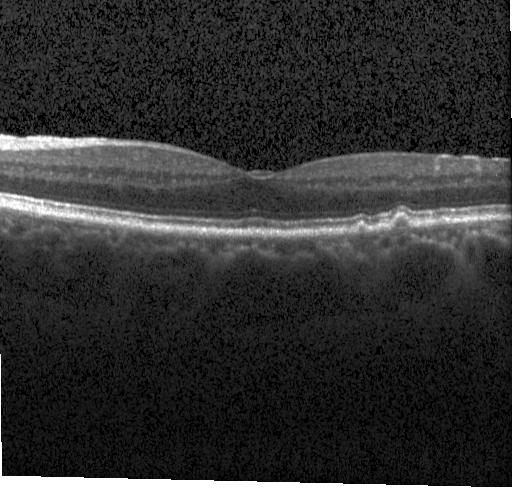

Acquired on a Heidelberg Spectralis, optical coherence tomography scan, through the macula. Impression: multiple drusen.